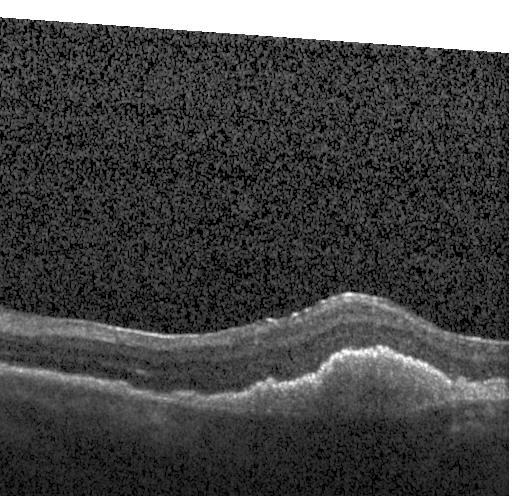 Diagnosis: CNV.